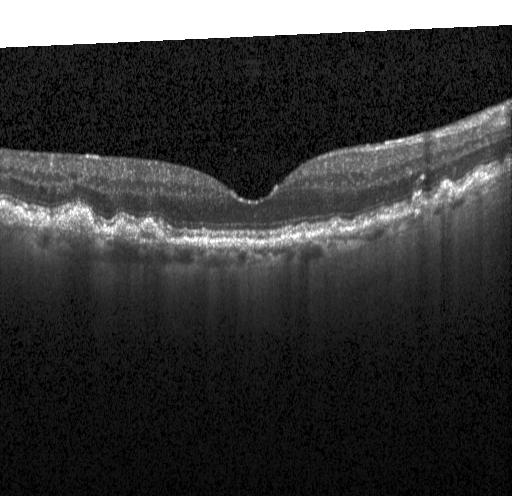 Optical coherence tomography B-scan, spectral-domain optical coherence tomography, acquired on a Heidelberg Spectralis — This B-scan demonstrates sub-RPE drusenoid deposits.